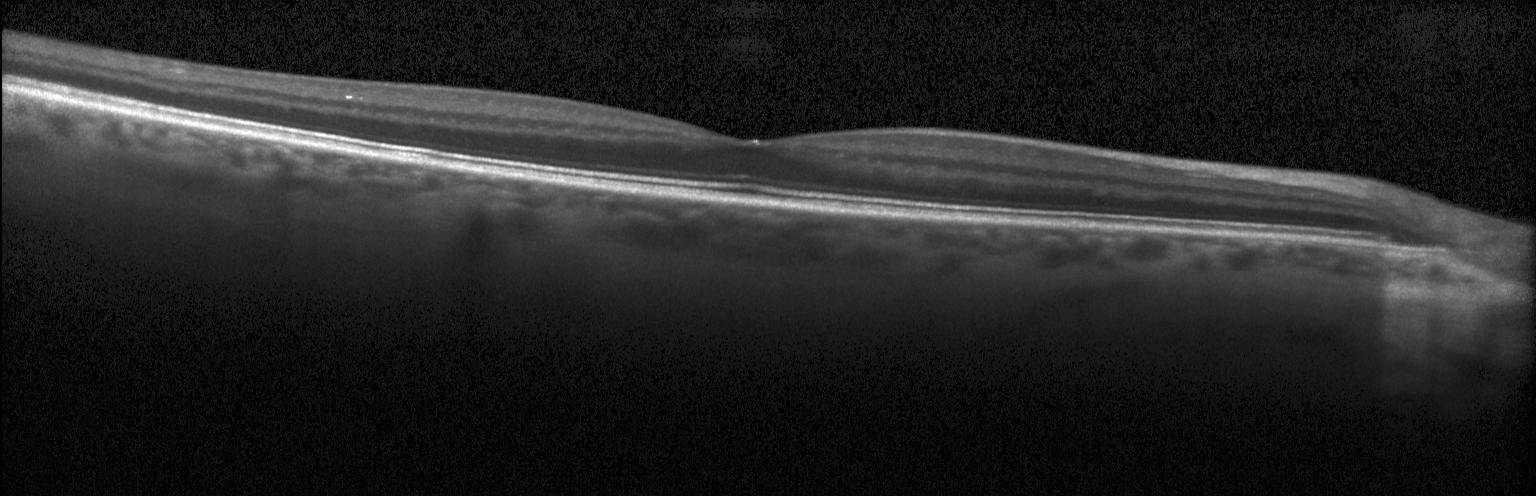

Through the macula, spectral-domain optical coherence tomography, Heidelberg Spectralis OCT system, OCT line scan — Assessment: no choroidal neovascularization, diabetic macular edema, or drusen.